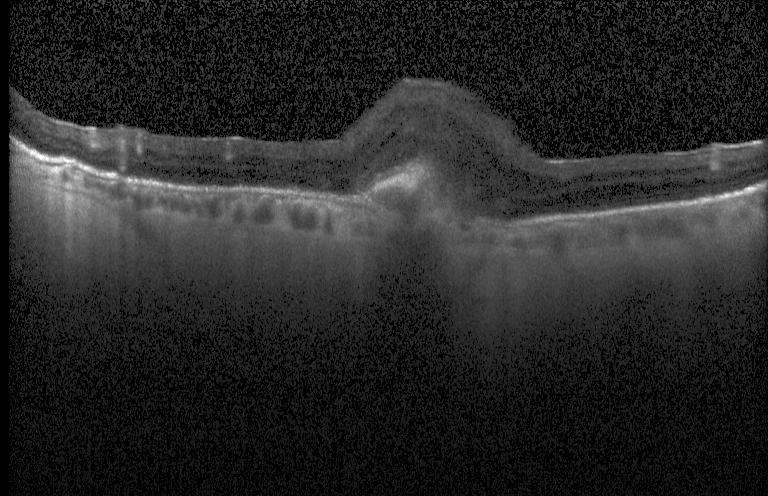 Optical coherence tomography scan — Dx: choroidal neovascularization.